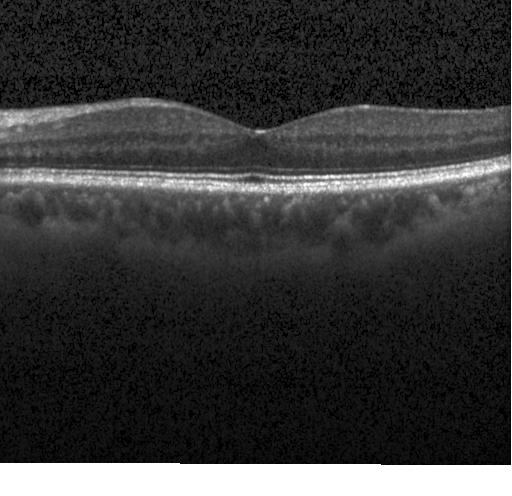
Assessment: no evidence of choroidal neovascularization, diabetic macular edema, or drusen.